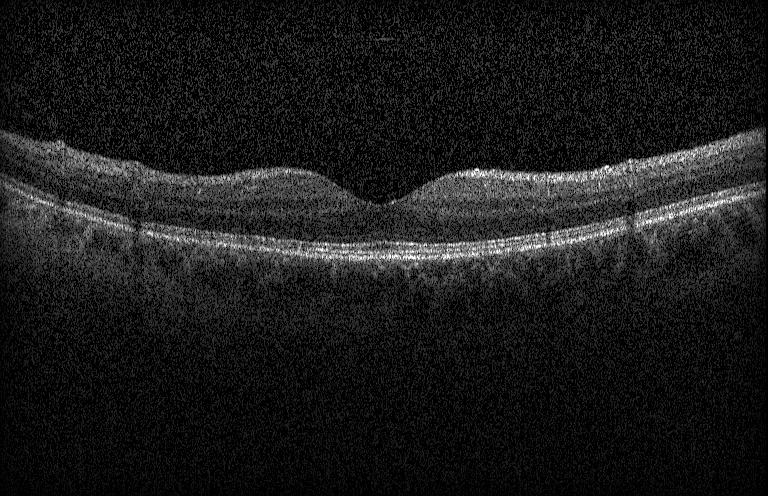

Diagnosis: no choroidal neovascularization, no diabetic macular edema, and no drusen.